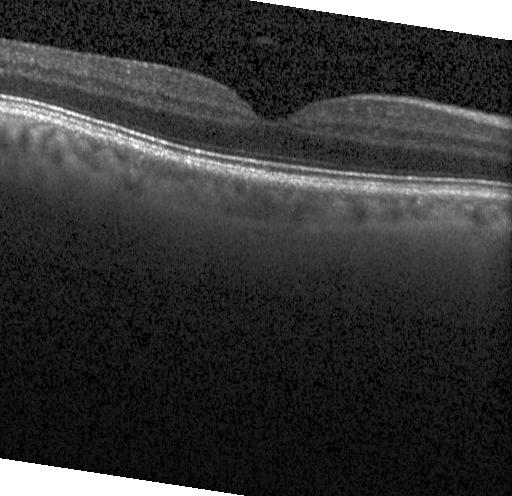 Finding: no choroidal neovascularization, no diabetic macular edema, and no drusen.